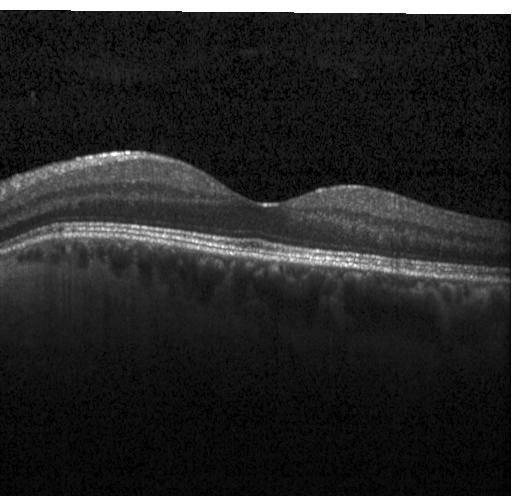 Finding: neither choroidal neovascularization, diabetic macular edema, nor drusen.